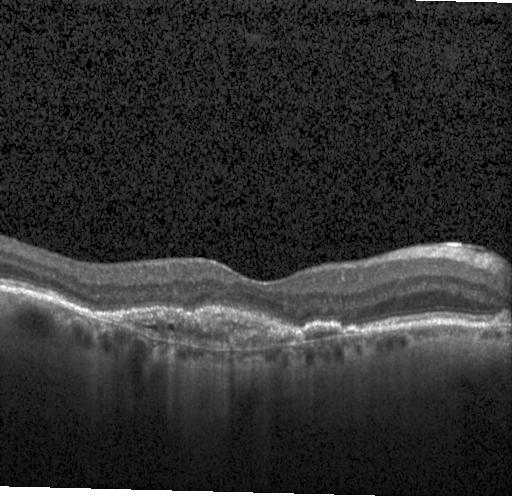

Diagnosis: a choroidal neovascular membrane.